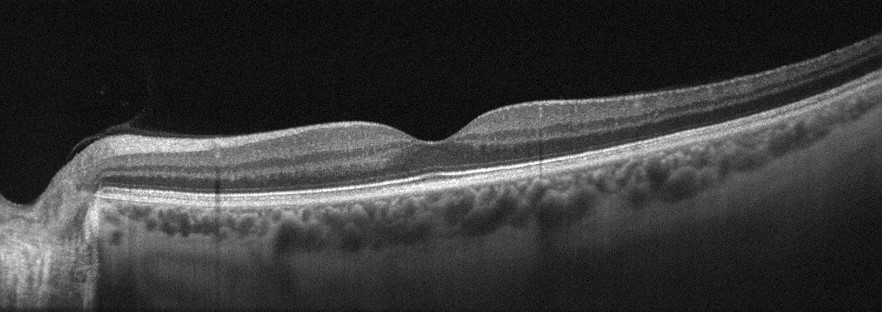 Retinal OCT cross-section showing no evidence of AMD, DME, ERM, RAO, RVO, or VID.